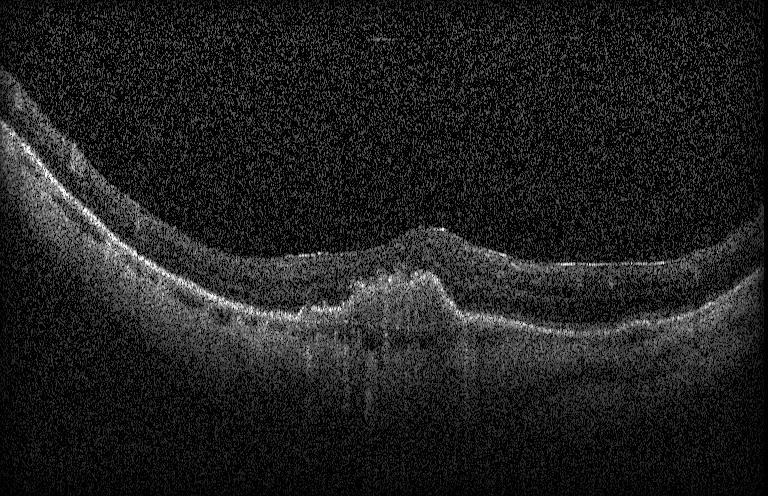

Instrument: Heidelberg Spectralis · optical coherence tomography scan · through the macula.
The scan shows CNV.